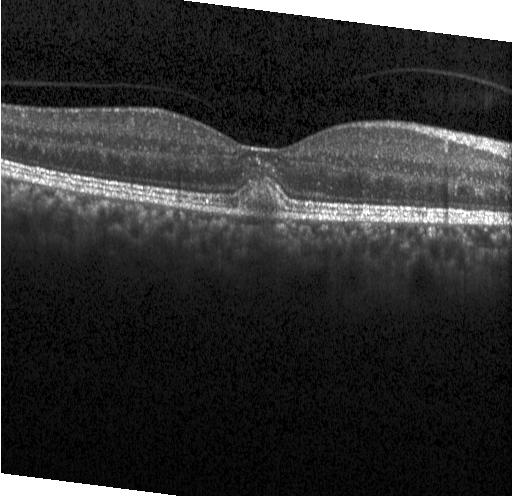 OCT scan showing a choroidal neovascular membrane.